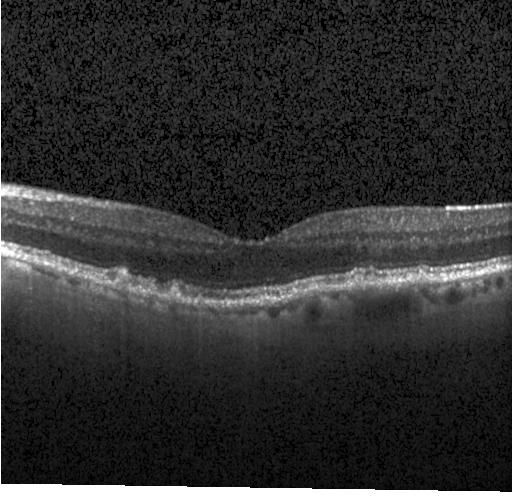

Optical coherence tomography B-scan. Heidelberg Spectralis — Dx: multiple drusen.